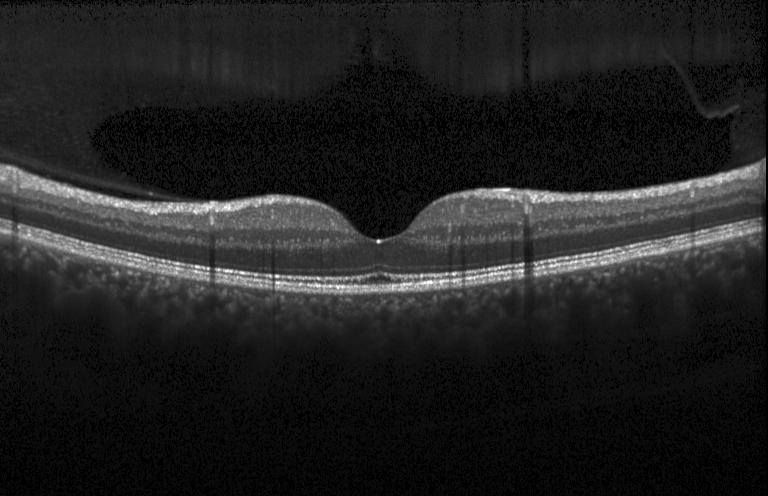 Optical coherence tomography scan. Heidelberg Spectralis. Centered on the fovea. Spectral-domain OCT.
Impression: neither CNV, DME, nor drusen.